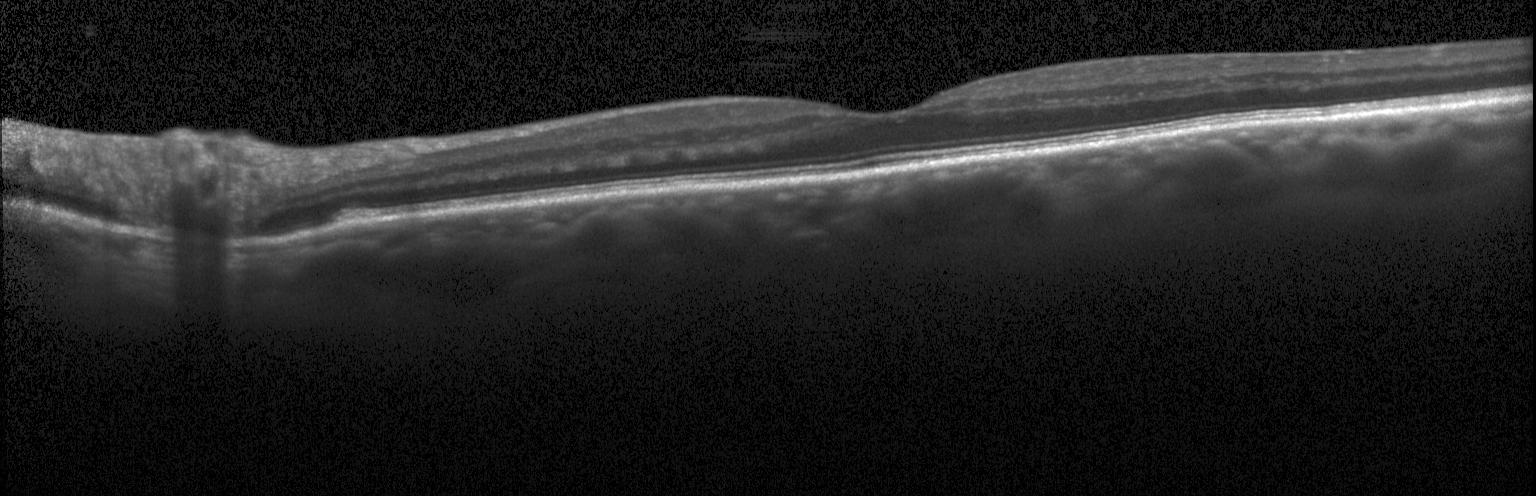 Spectral-domain OCT B-scan: no choroidal neovascularization, no diabetic macular edema, and no drusen.